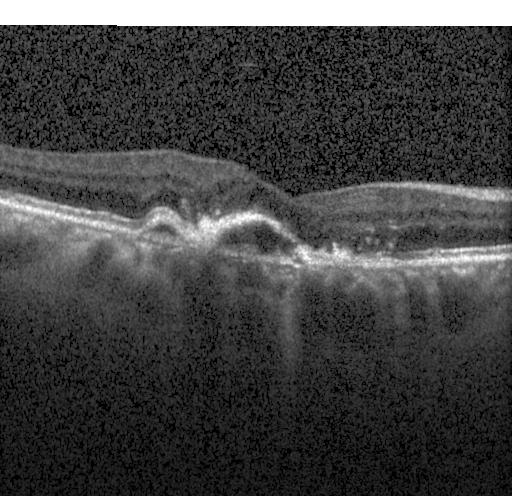 Retinal OCT B-scan. Assessment: choroidal neovascularization (CNV).